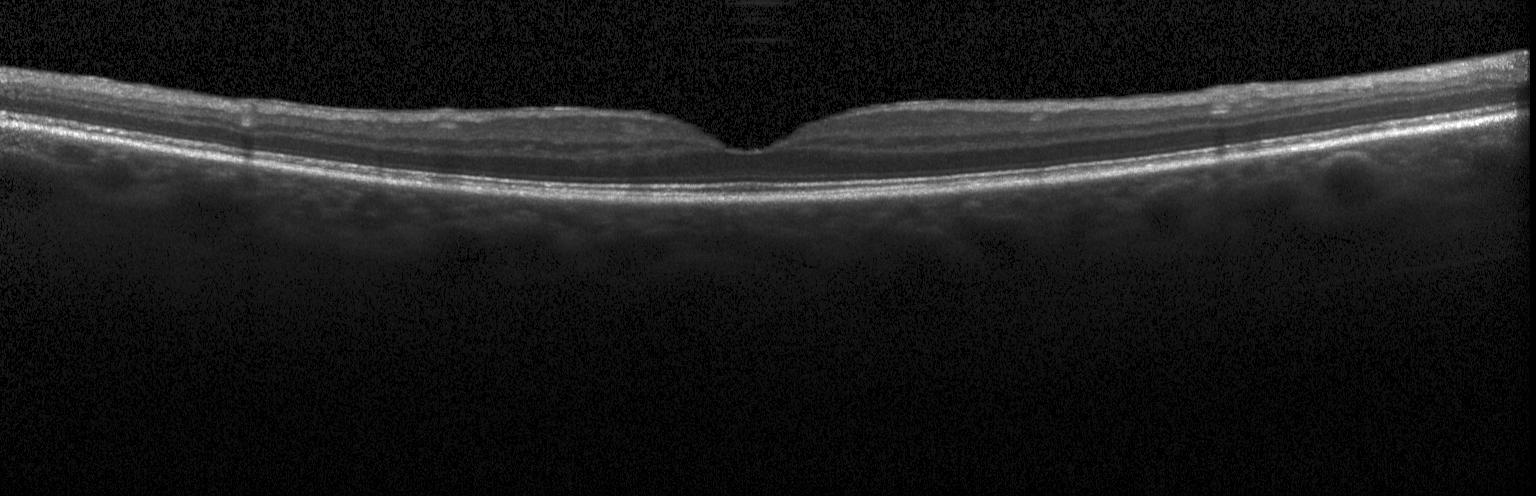

Macular OCT: no choroidal neovascularization, no diabetic macular edema, and no drusen.